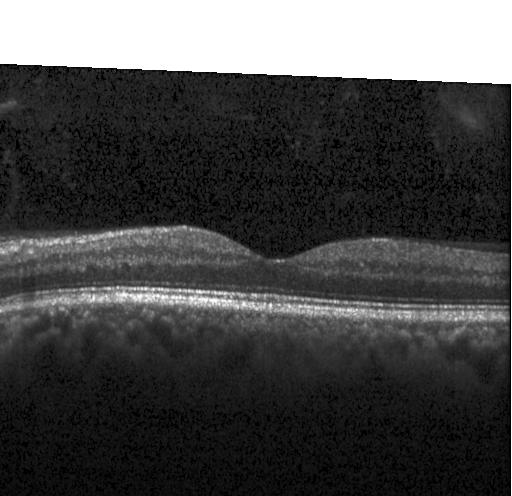 Macular OCT: no choroidal neovascularization, diabetic macular edema, or drusen.